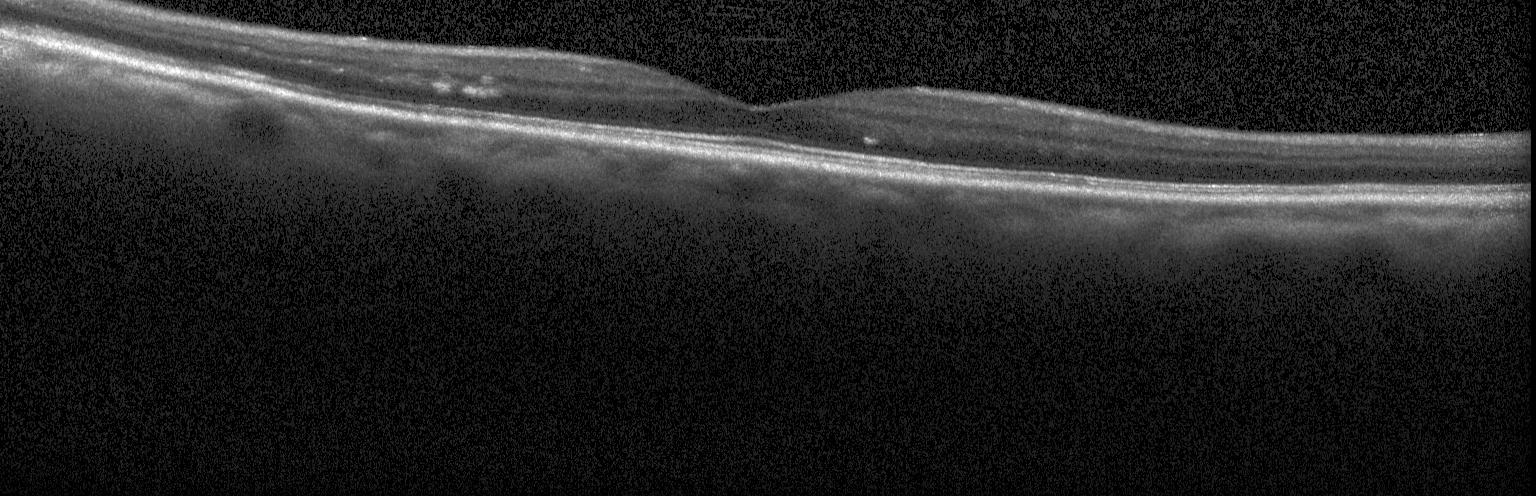 Retinal OCT cross-section. Macular scan. Acquired on a Heidelberg Spectralis. Spectral-domain OCT. No evidence of CNV, DME, or drusen.